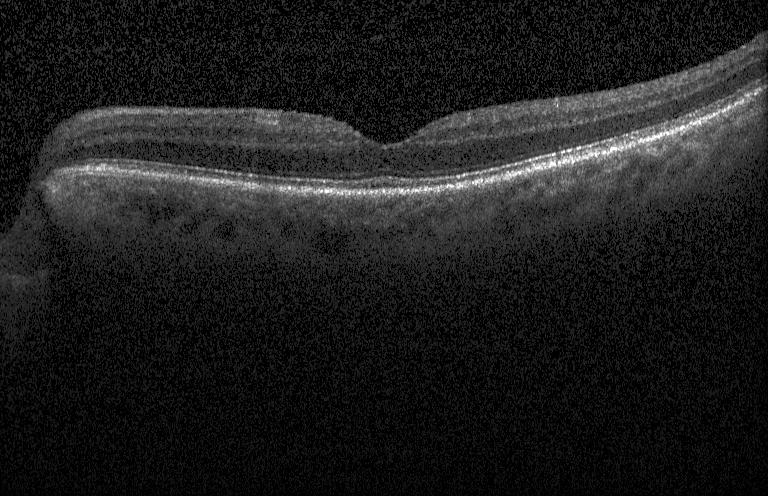 OCT B-scan. Acquired on a Heidelberg Spectralis. Finding: neither CNV, DME, nor drusen.